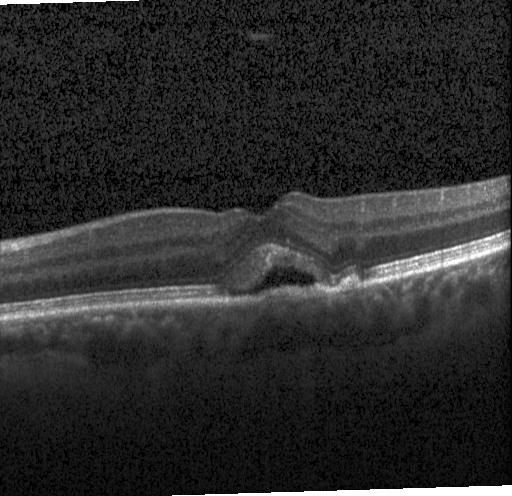
Spectral-domain optical coherence tomography · centered on the fovea · instrument: Heidelberg Spectralis · optical coherence tomography B-scan — Impression: CNV.